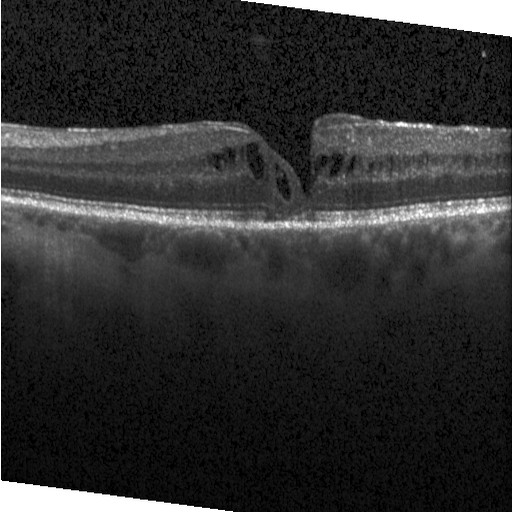 Retinal OCT cross-section, macular scan, spectral-domain OCT — Assessment: DME.